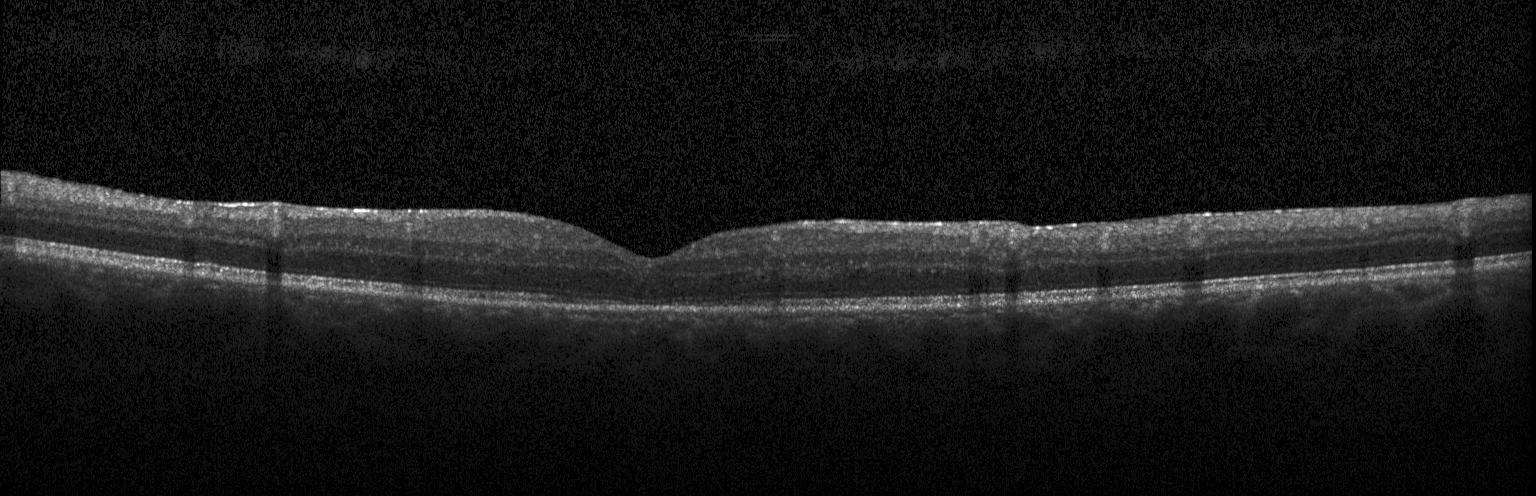
Instrument: Heidelberg Spectralis · spectral-domain optical coherence tomography · OCT line scan.
Impression: no choroidal neovascularization, diabetic macular edema, or drusen.